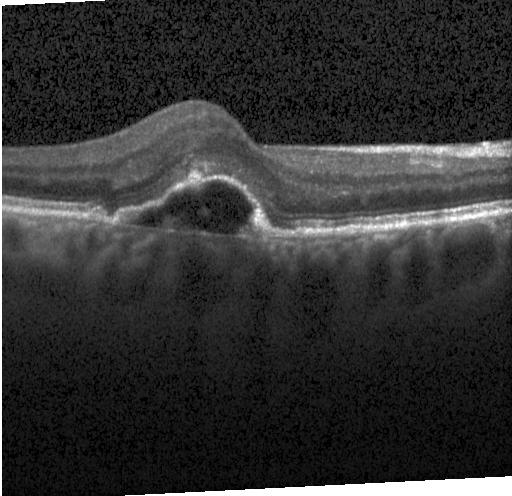
Optical coherence tomography scan. Acquired on a Heidelberg Spectralis. Finding: choroidal neovascularization (CNV).